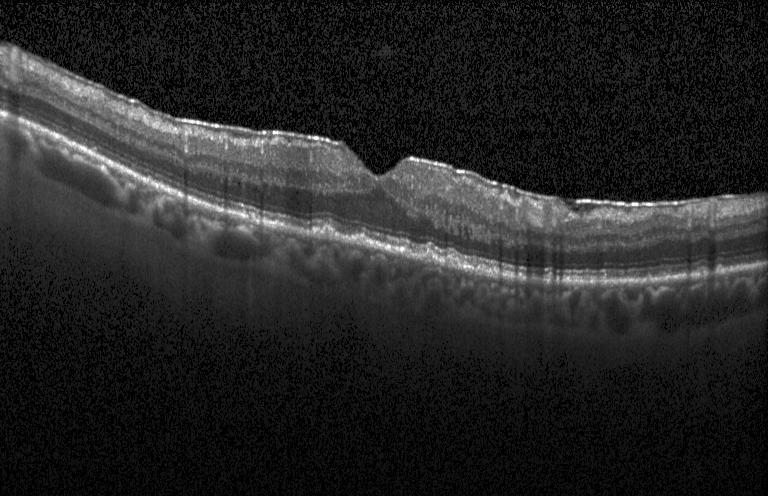

Instrument: Heidelberg Spectralis, horizontal scan through the fovea, optical coherence tomography scan, spectral-domain OCT
Diagnosis: multiple drusen.